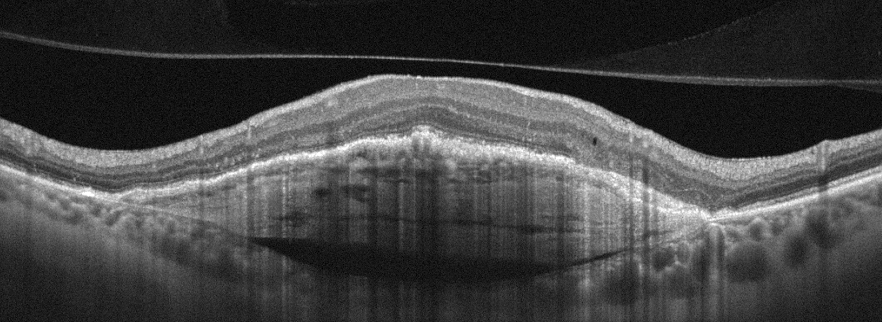
Fovea-centered · OCT B-scan. Impression: age-related macular degeneration (AMD).